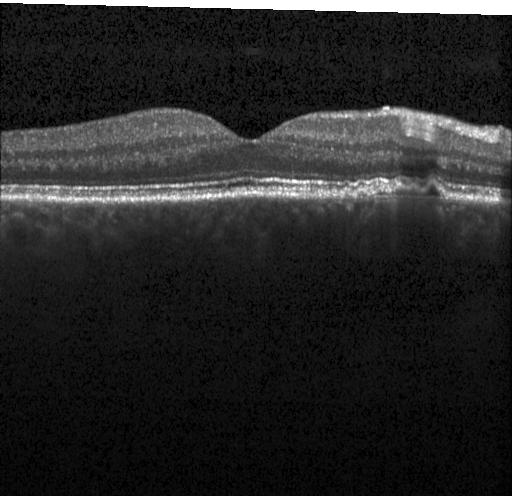

Optical coherence tomography scan — This B-scan demonstrates a choroidal neovascular membrane.